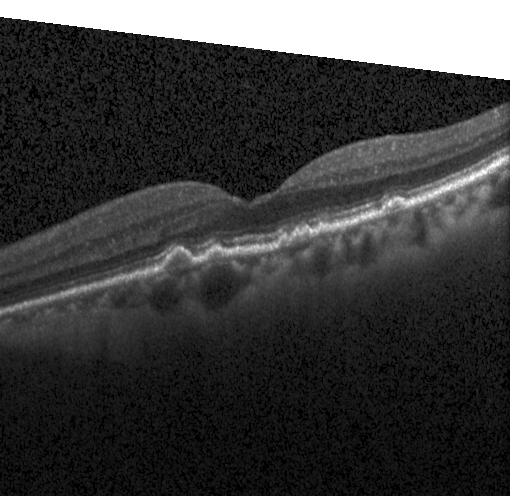
Instrument: Heidelberg Spectralis · OCT line scan — Dx: multiple drusen.